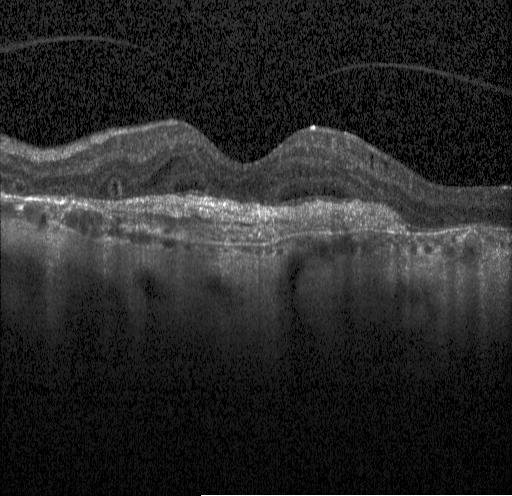

Retinal OCT B-scan; Heidelberg Spectralis. The scan shows a choroidal neovascular membrane.